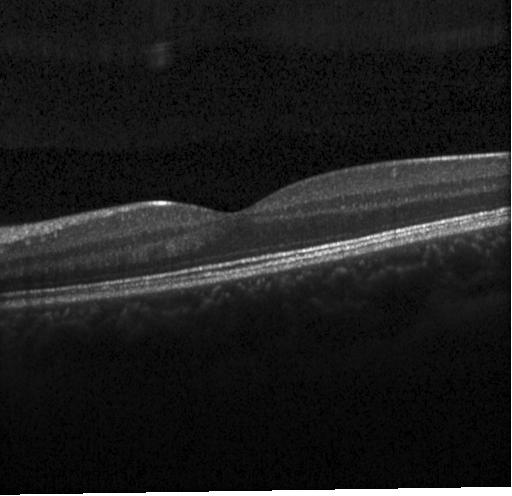

Optical coherence tomography scan. OCT finding: no CNV, no DME, and no drusen.